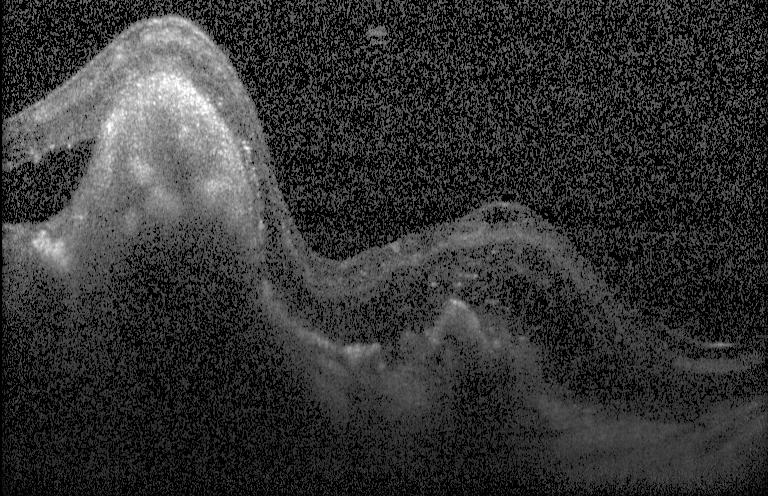

Optical coherence tomography B-scan, spectral-domain OCT, acquired on a Heidelberg Spectralis. The scan shows CNV.